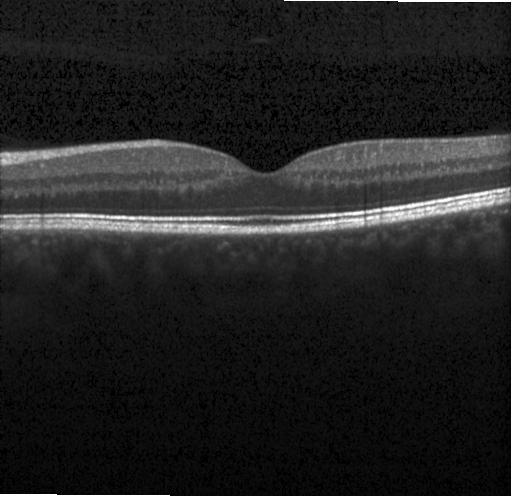

Optical coherence tomography scan. Centered on the fovea. SD-OCT. Acquired on a Heidelberg Spectralis
Assessment: no choroidal neovascularization, diabetic macular edema, or drusen.